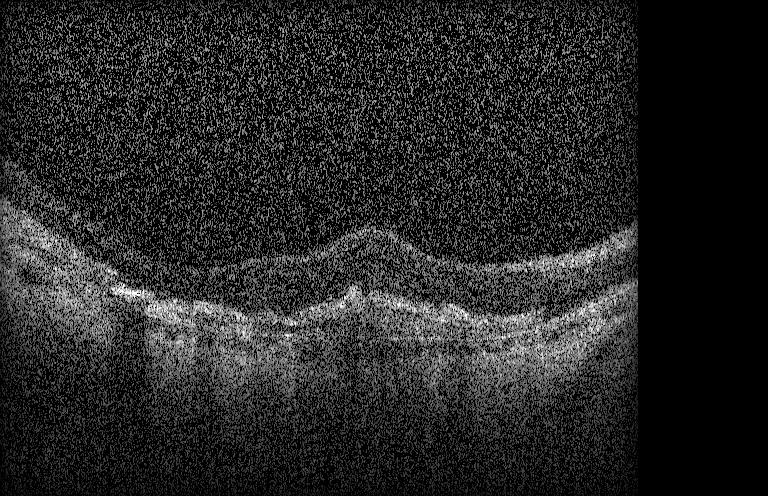
Retinal OCT cross-section showing a choroidal neovascular membrane.